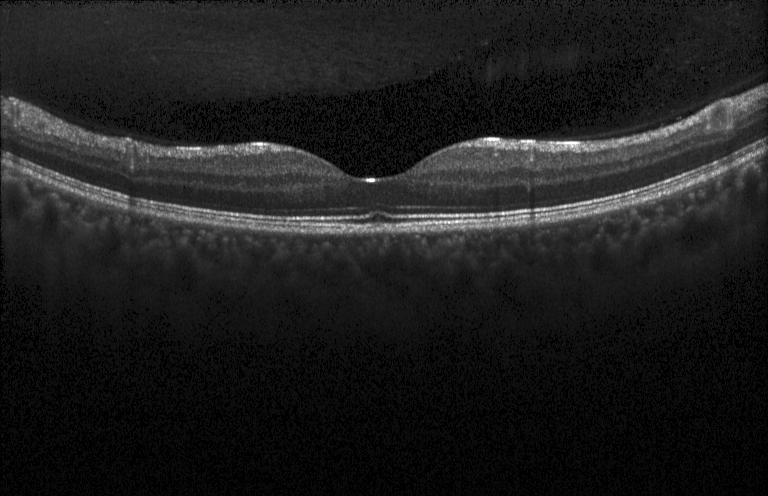

Spectral-domain OCT. OCT line scan.
Diagnosis: no evidence of CNV, DME, or drusen.